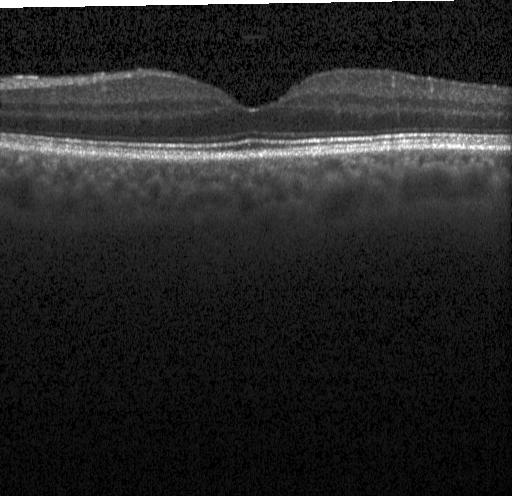 Spectral-domain OCT · OCT B-scan · Heidelberg Spectralis · through the macula. Dx: no evidence of CNV, DME, or drusen.